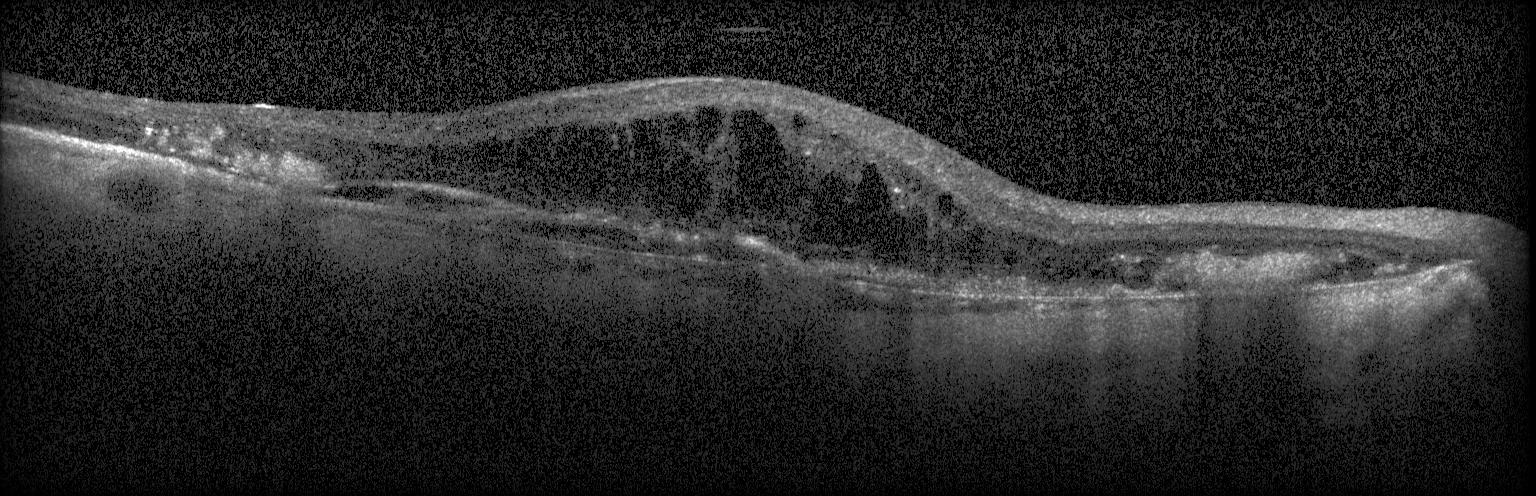
OCT B-scan, macular scan.
Impression: choroidal neovascularization (CNV).